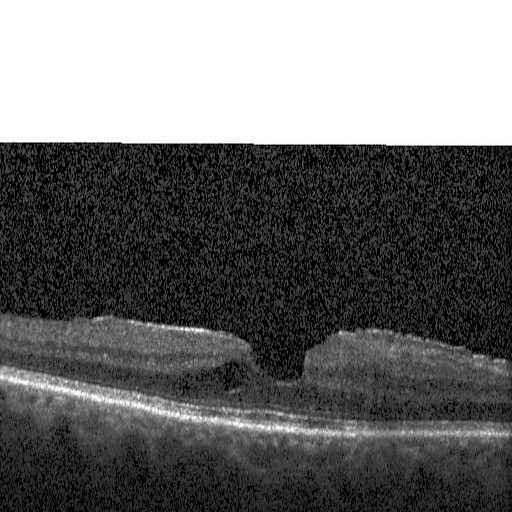 OCT finding: diabetic macular edema (DME).